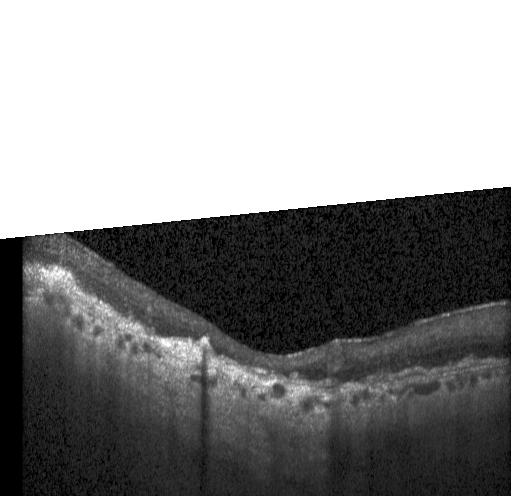 Spectral-domain optical coherence tomography; optical coherence tomography scan. Diagnosis: a choroidal neovascular membrane.